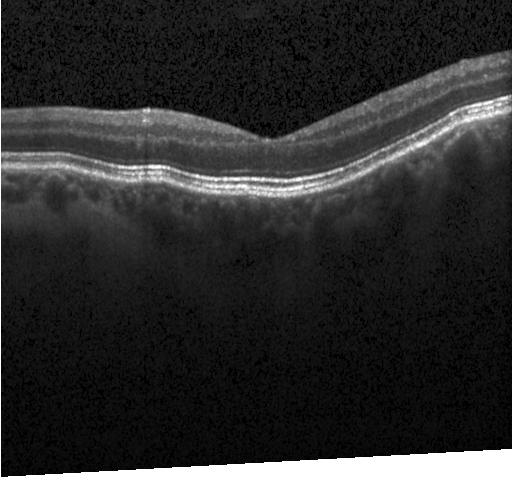
Macular OCT: no choroidal neovascularization, diabetic macular edema, or drusen.